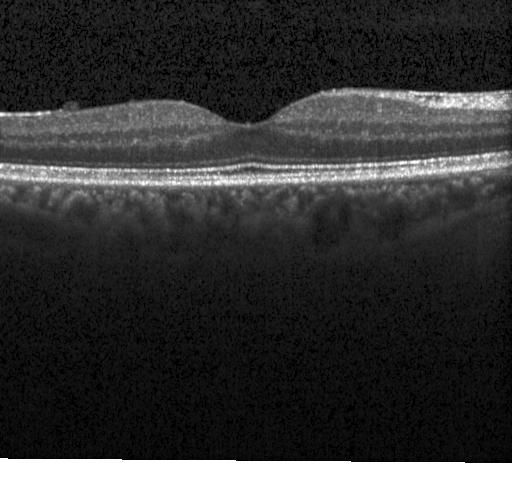

Retinal OCT B-scan. Spectral-domain optical coherence tomography.
OCT finding: neither choroidal neovascularization, diabetic macular edema, nor drusen.